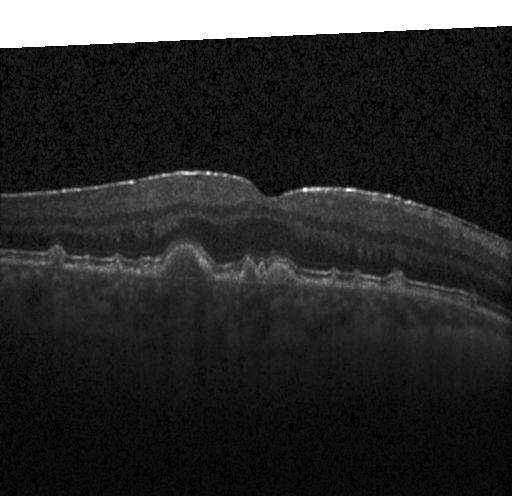

Retinal OCT B-scan — Choroidal neovascularization (CNV).